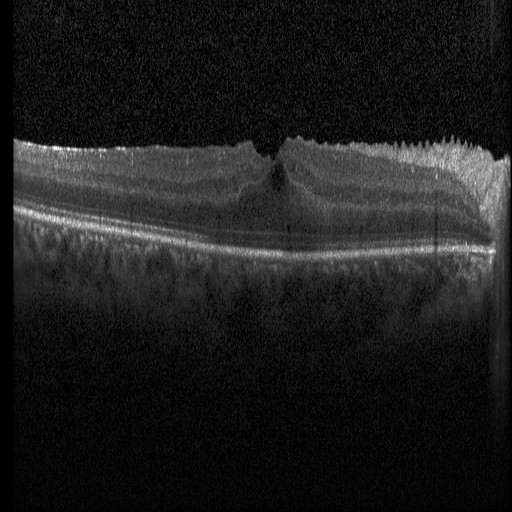 Macular scan. Acquired on a Heidelberg Spectralis. Optical coherence tomography B-scan
Finding: diabetic macular edema (DME).